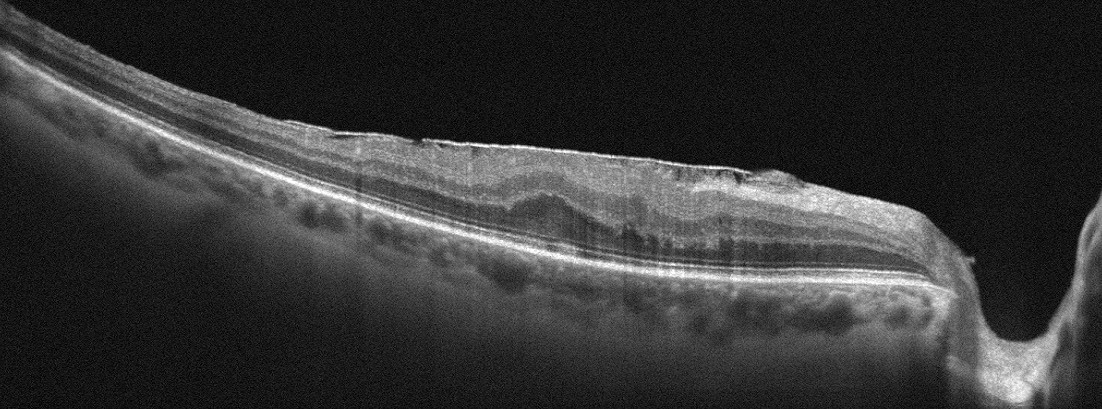 Optical coherence tomography scan
Assessment: ERM.